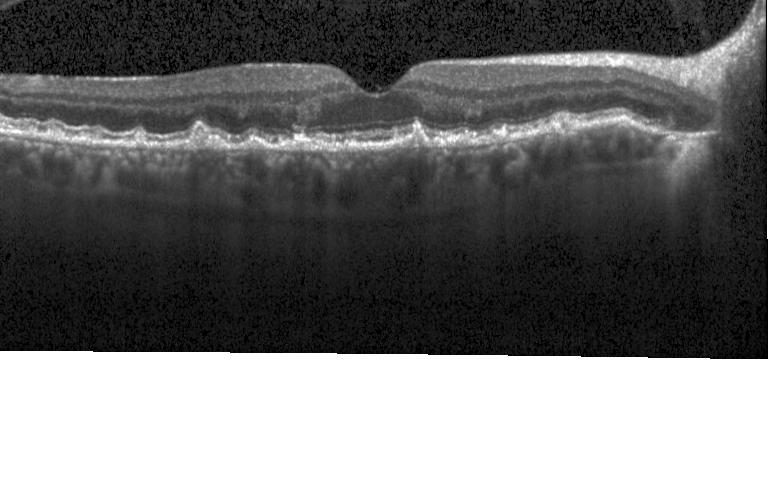

Optical coherence tomography B-scan
Impression: drusen.